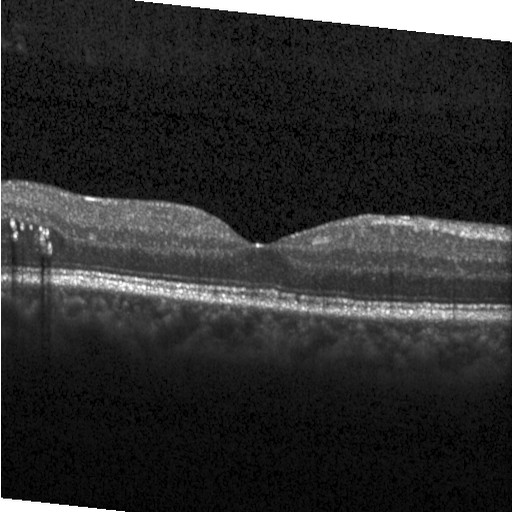 DME.